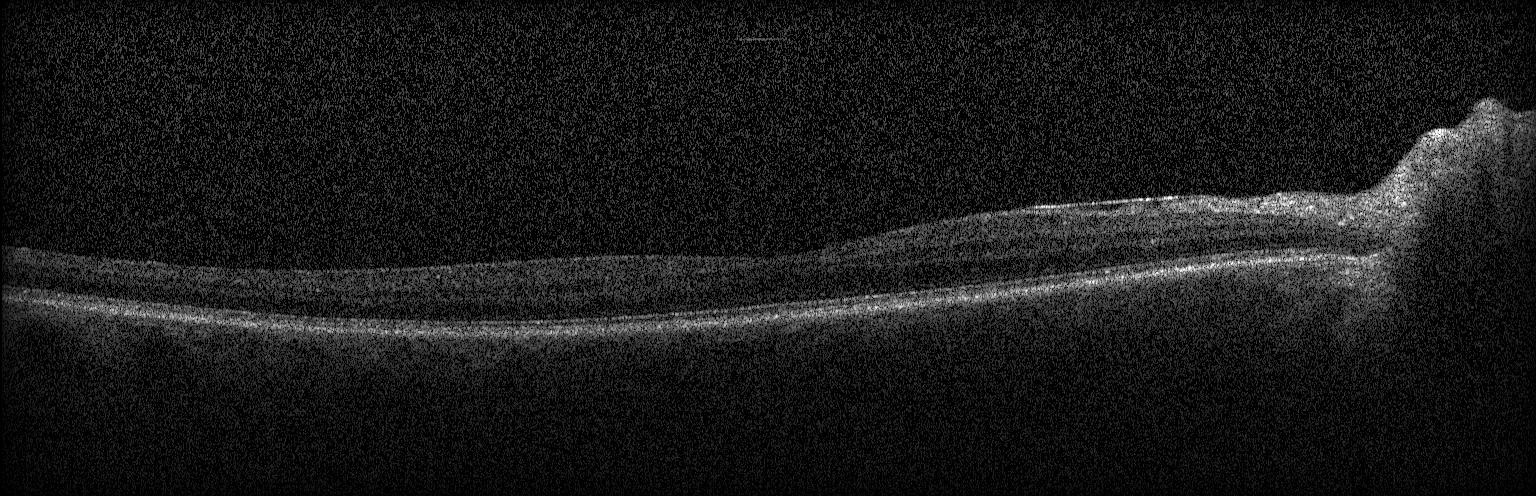

No choroidal neovascularization, diabetic macular edema, or drusen.